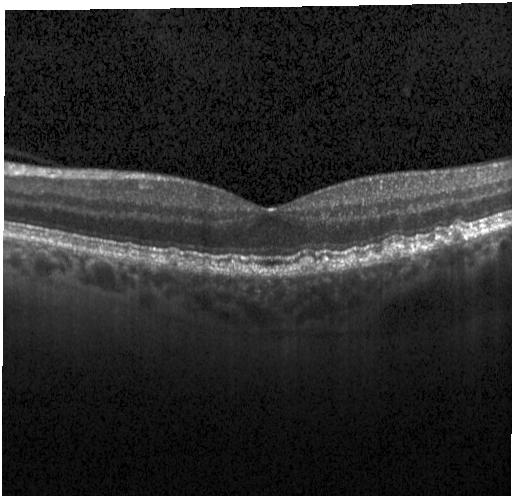
Sub-RPE drusenoid deposits.